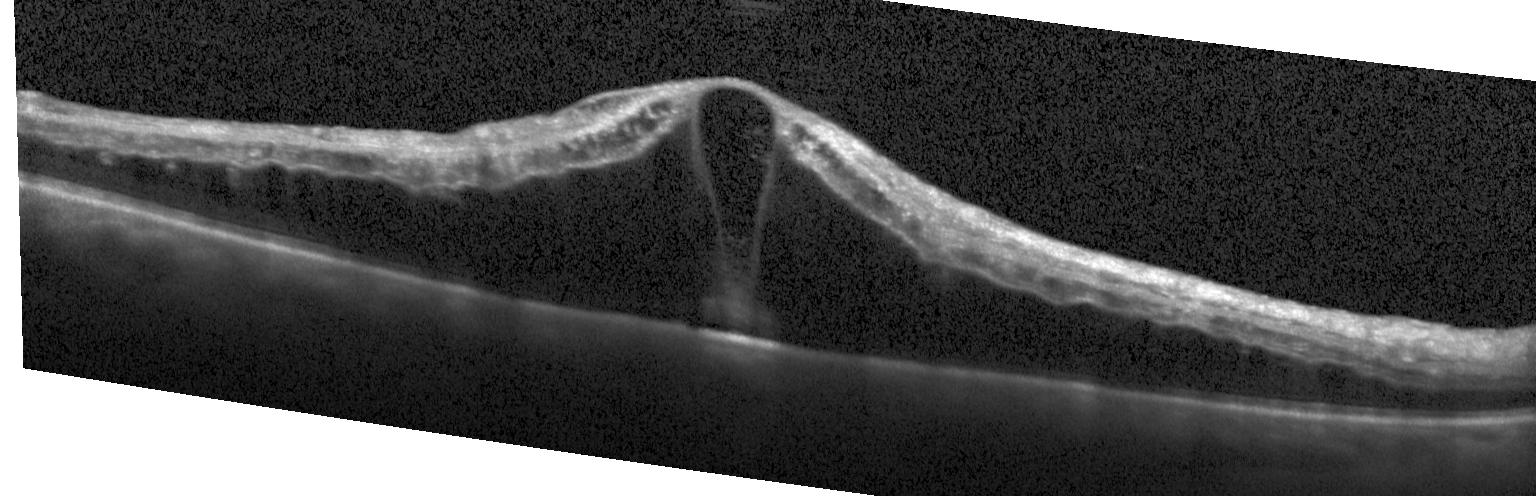
OCT B-scan showing DME.